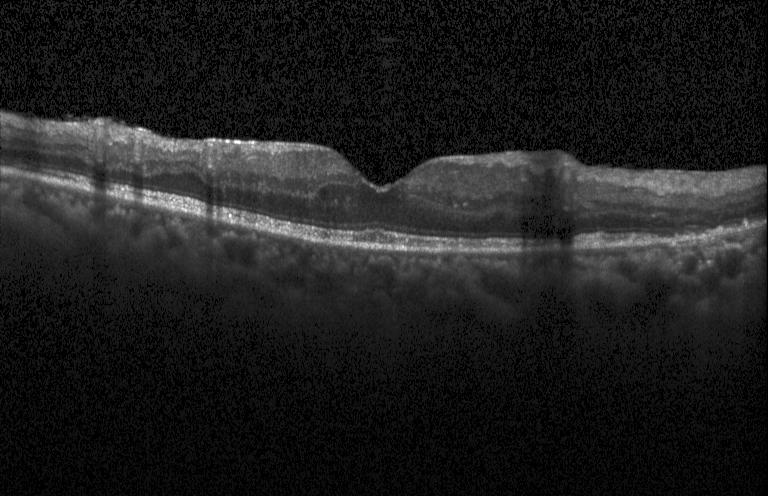

Acquired on a Heidelberg Spectralis. Centered on the fovea. Retinal OCT B-scan. Spectral-domain OCT.
This B-scan demonstrates diabetic macular edema (DME).